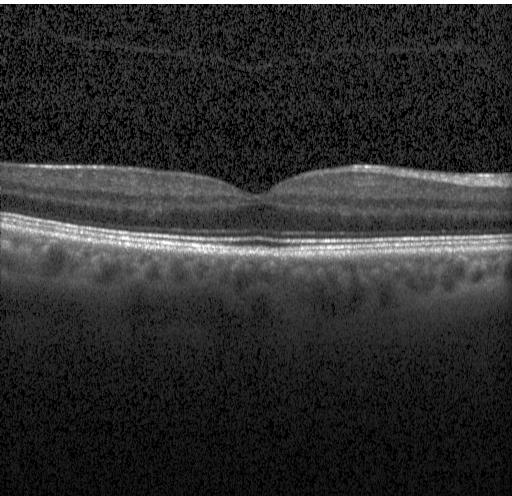

Instrument: Heidelberg Spectralis; spectral-domain OCT; optical coherence tomography scan — No choroidal neovascularization, no diabetic macular edema, and no drusen.